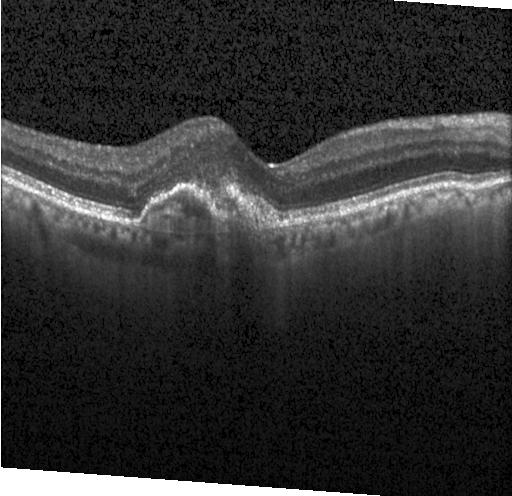
OCT B-scan — Impression: CNV.